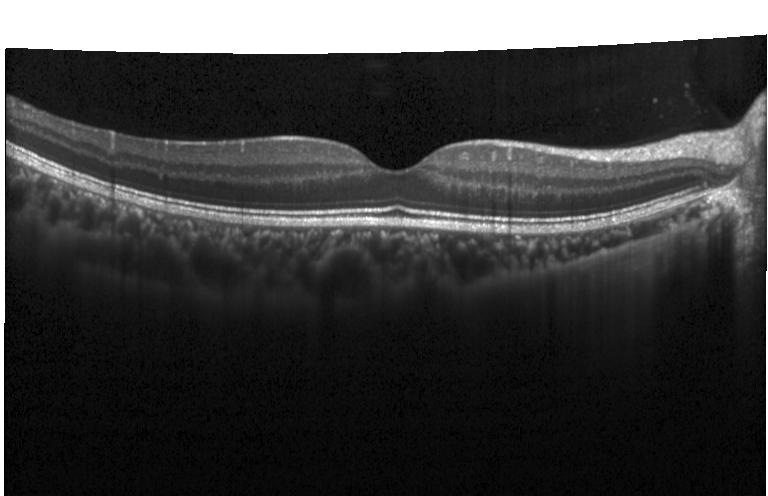
Spectral-domain OCT B-scan: no evidence of choroidal neovascularization, diabetic macular edema, or drusen.